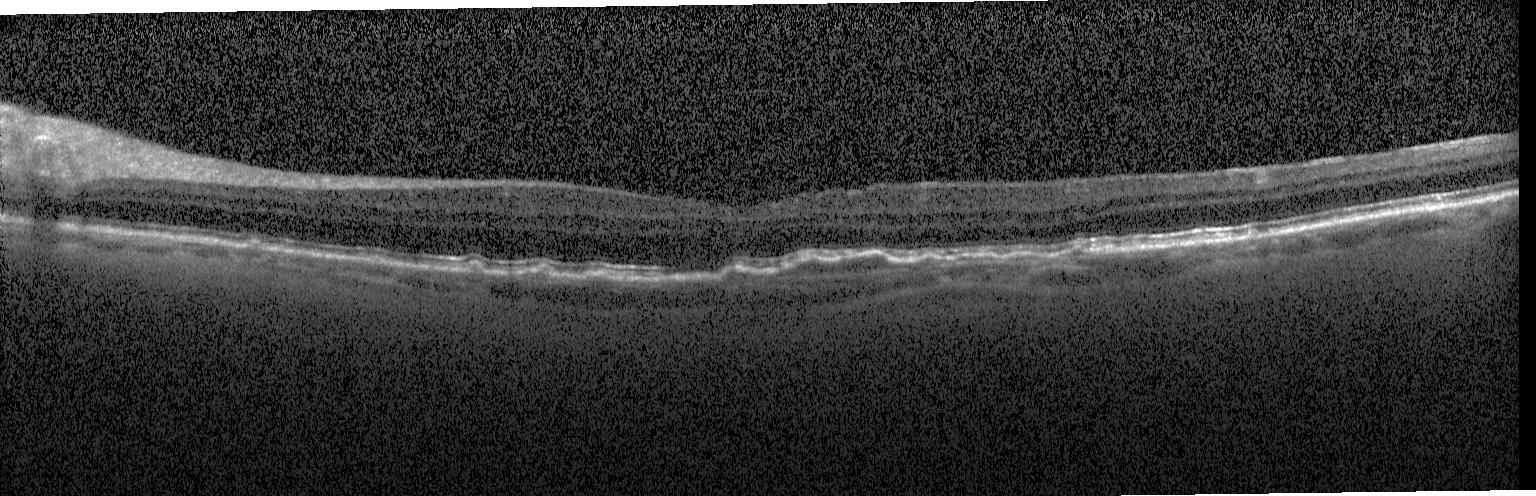

Optical coherence tomography B-scan.
Macular OCT: multiple drusen.